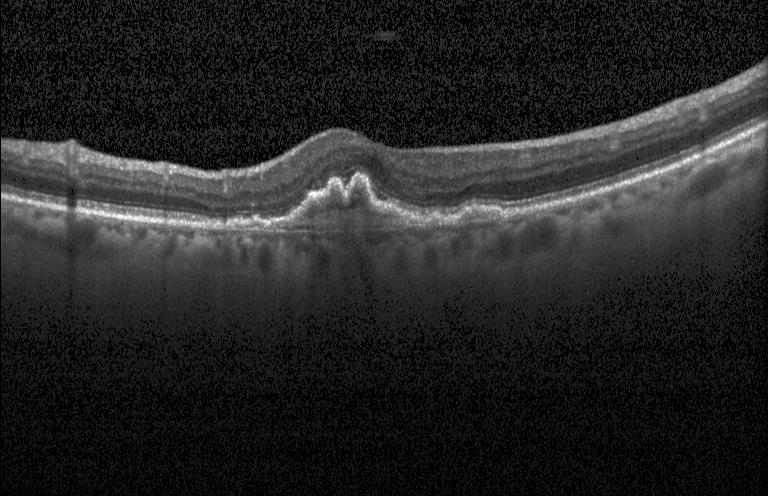

OCT scan showing a choroidal neovascular membrane.